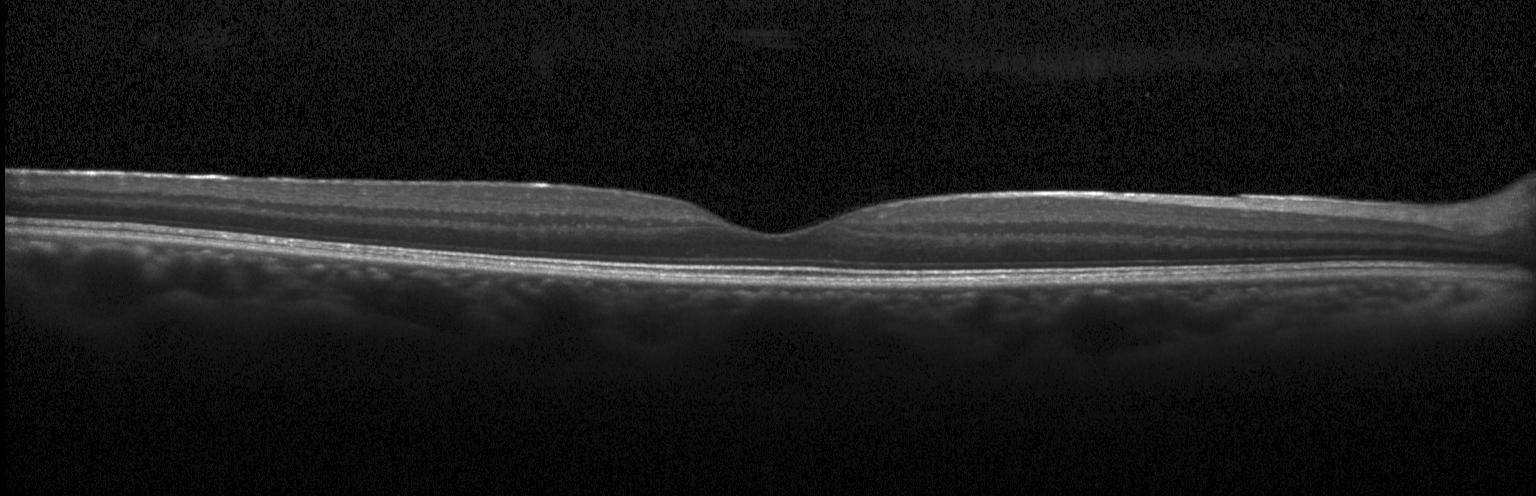

OCT B-scan.
No CNV, DME, or drusen.